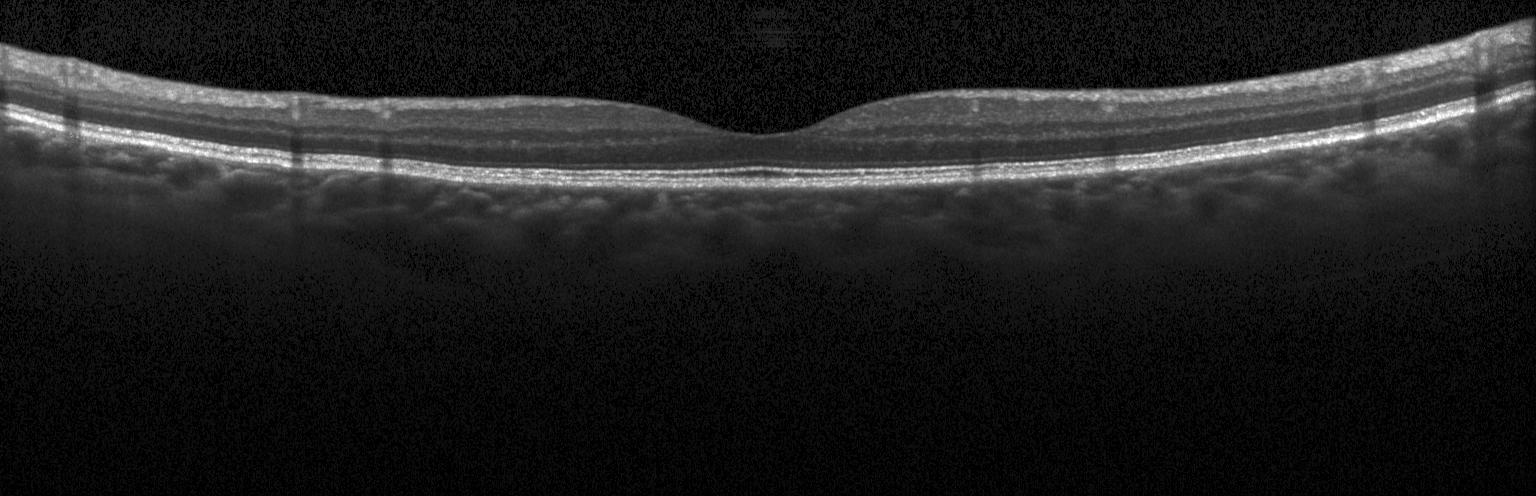 Heidelberg Spectralis. Spectral-domain optical coherence tomography. Through the macula. Retinal OCT B-scan
No evidence of choroidal neovascularization, diabetic macular edema, or drusen.